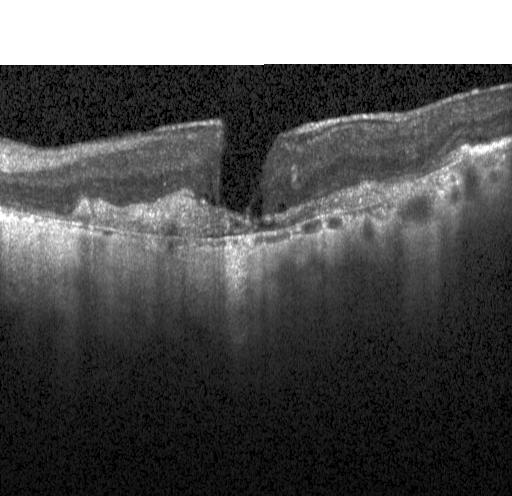
Instrument: Heidelberg Spectralis · optical coherence tomography scan · spectral-domain optical coherence tomography
Diagnosis: CNV.